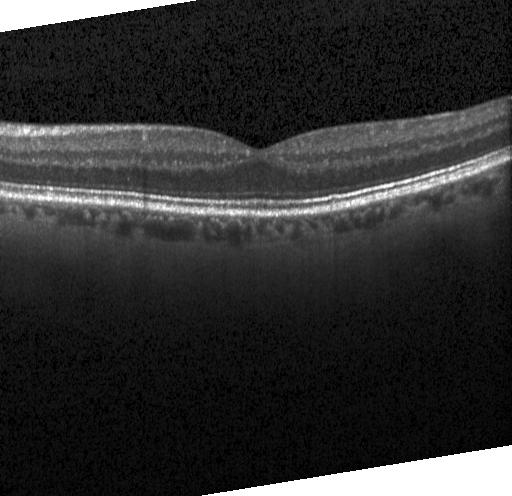 Through the macula, spectral-domain OCT, acquired on a Heidelberg Spectralis, retinal OCT B-scan.
This B-scan demonstrates neither choroidal neovascularization, diabetic macular edema, nor drusen.